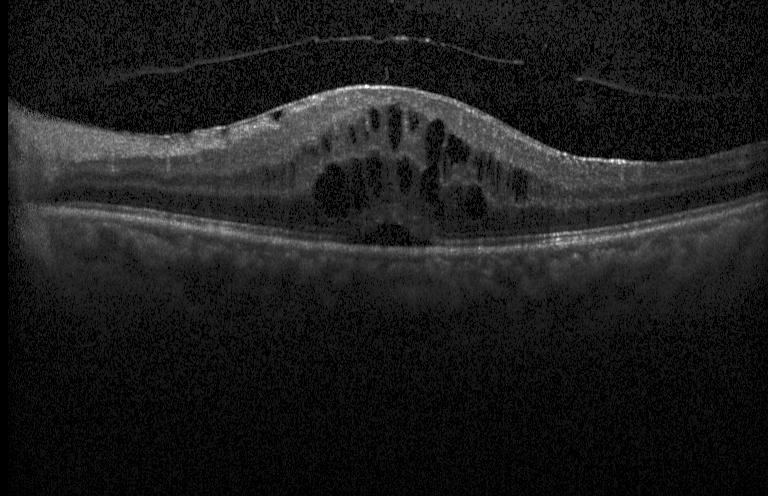
OCT line scan. Diagnosis: DME.